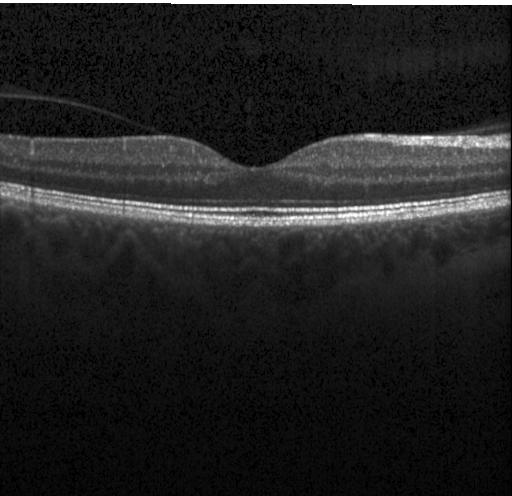

Macular OCT demonstrating no CNV, no DME, and no drusen.